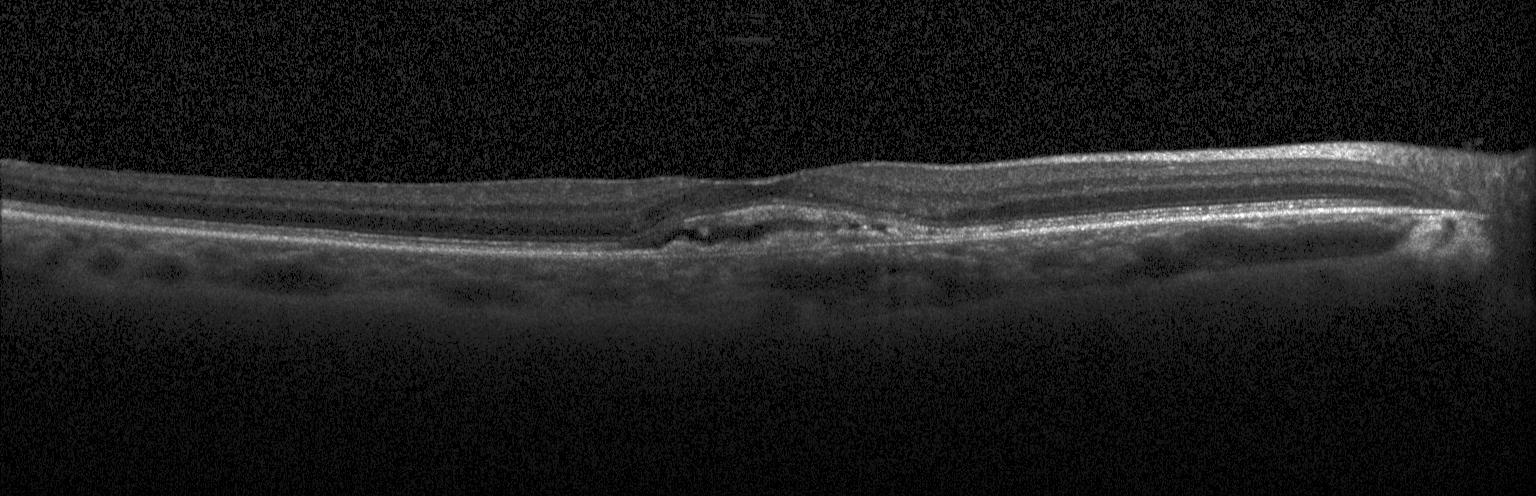 Macular OCT: CNV.